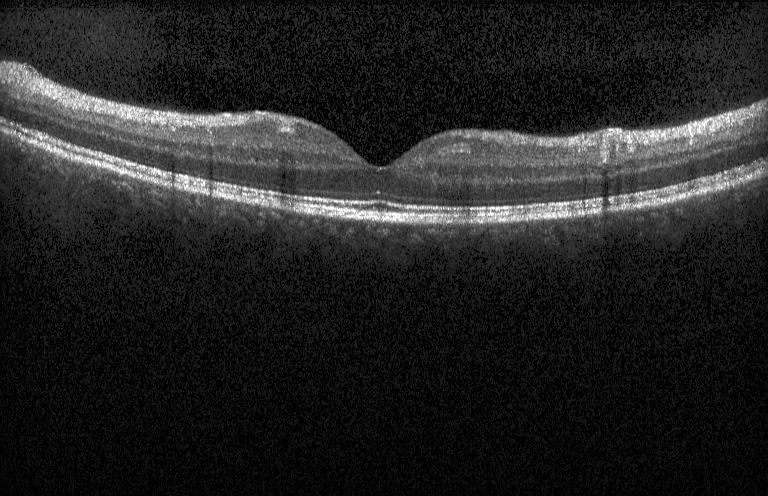

Dx: no choroidal neovascularization, no diabetic macular edema, and no drusen.